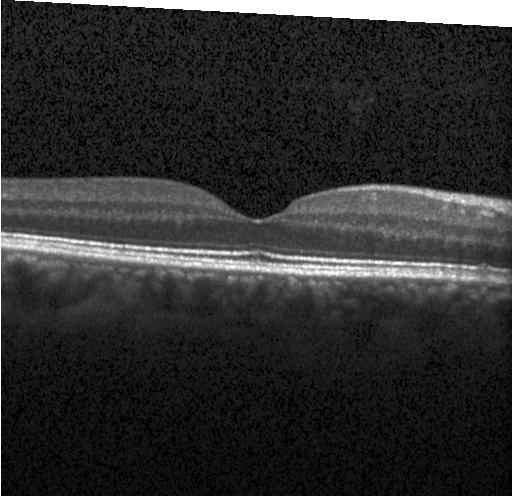 OCT scan showing neither choroidal neovascularization, diabetic macular edema, nor drusen.